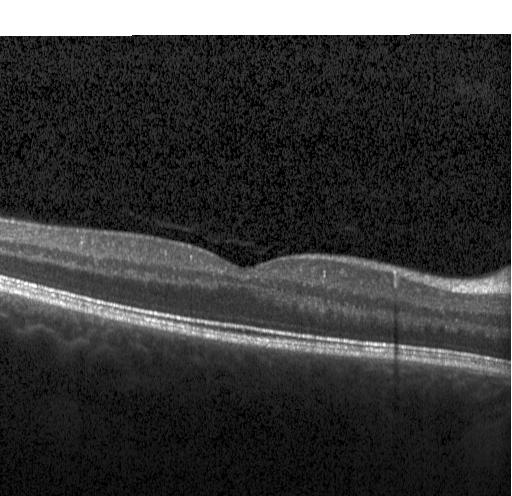
OCT scan showing neither choroidal neovascularization, diabetic macular edema, nor drusen.